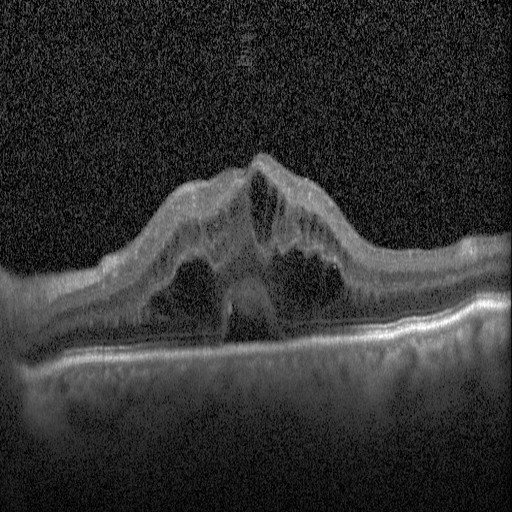
OCT line scan. The scan shows DME.